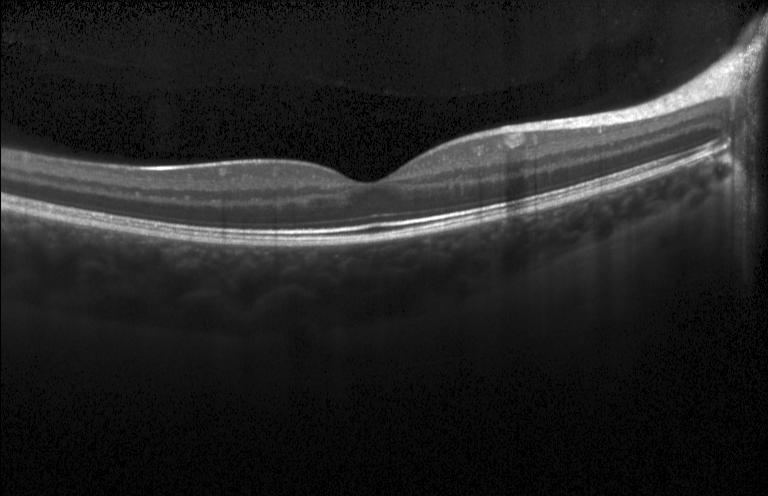
Acquired on a Heidelberg Spectralis; spectral-domain optical coherence tomography; macular scan; OCT B-scan. No evidence of choroidal neovascularization, diabetic macular edema, or drusen.